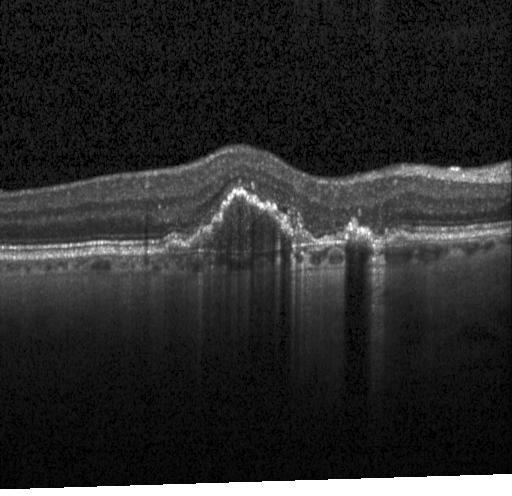 Finding: CNV.